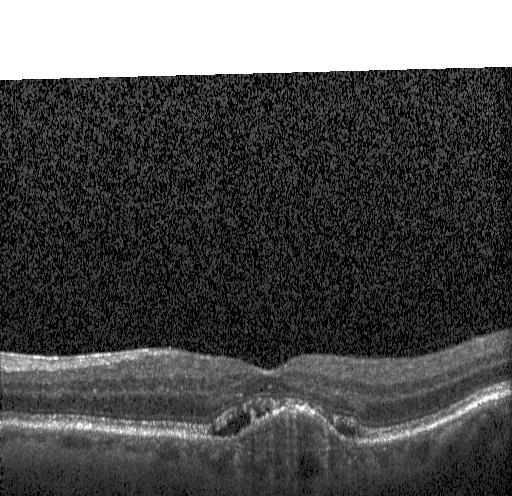 Retinal OCT cross-section. Impression: a choroidal neovascular membrane.